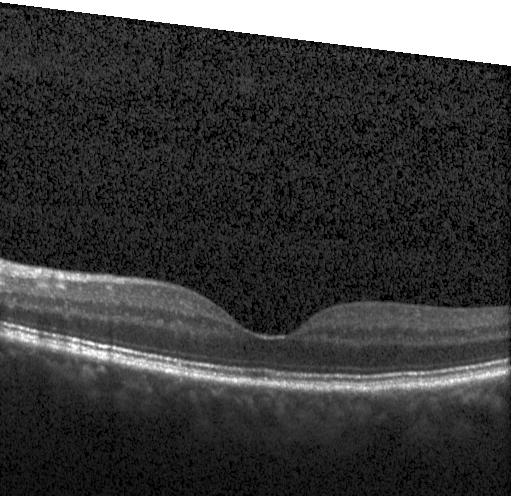

Retinal OCT B-scan, Heidelberg Spectralis — This B-scan demonstrates neither choroidal neovascularization, diabetic macular edema, nor drusen.